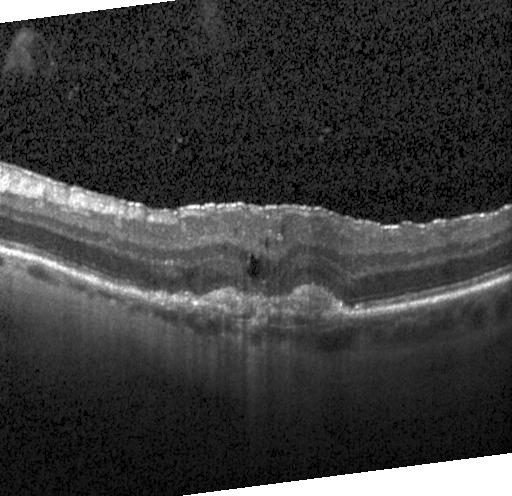

OCT finding: choroidal neovascularization.